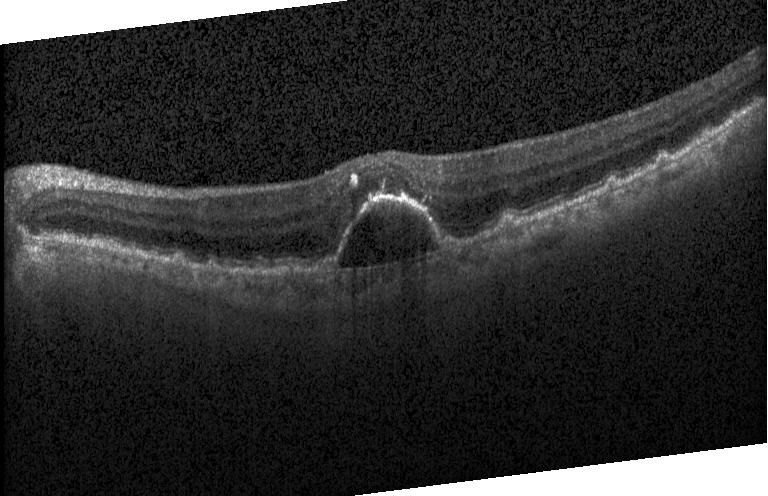

Macular OCT: CNV.